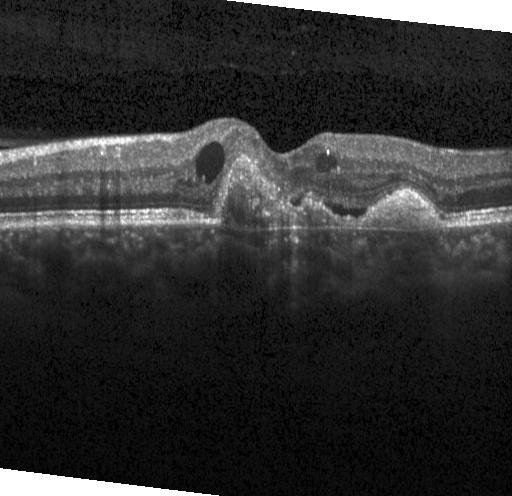 A choroidal neovascular membrane.